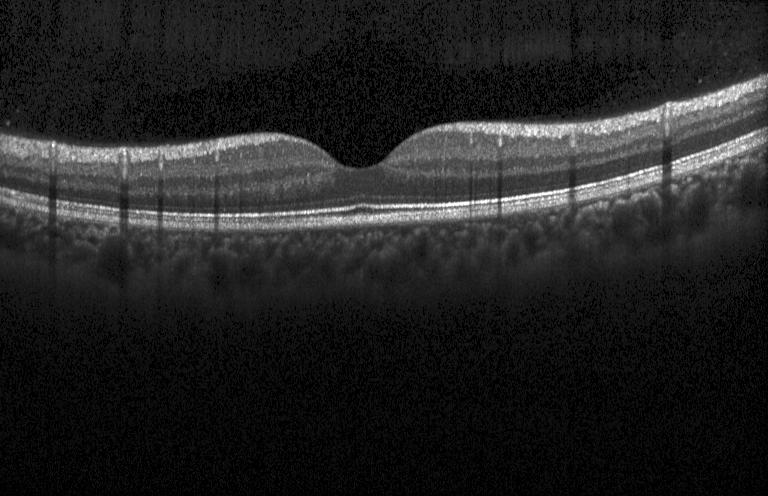

Finding: no evidence of CNV, DME, or drusen.